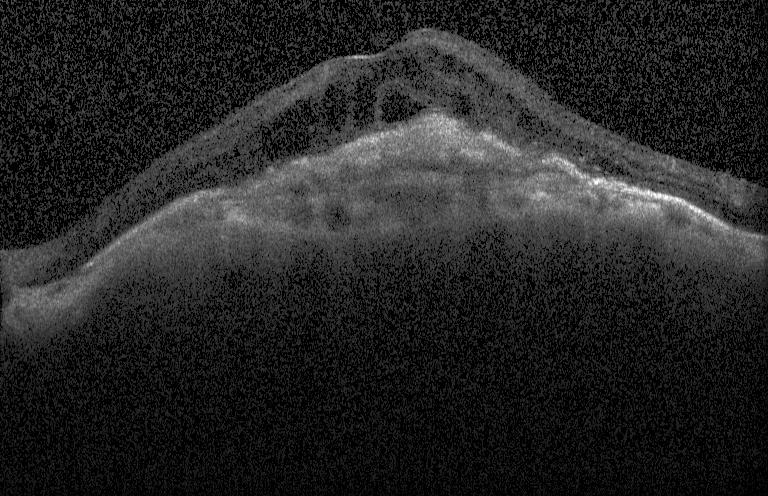

Optical coherence tomography B-scan. Fovea-centered.
Dx: a choroidal neovascular membrane.